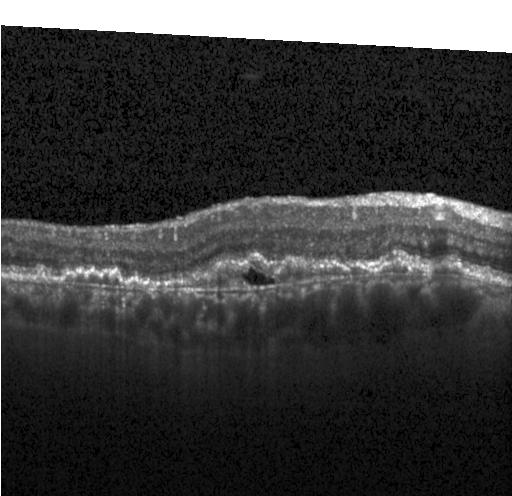 Fovea-centered, spectral-domain optical coherence tomography, acquired on a Heidelberg Spectralis, OCT B-scan.
Finding: choroidal neovascularization.